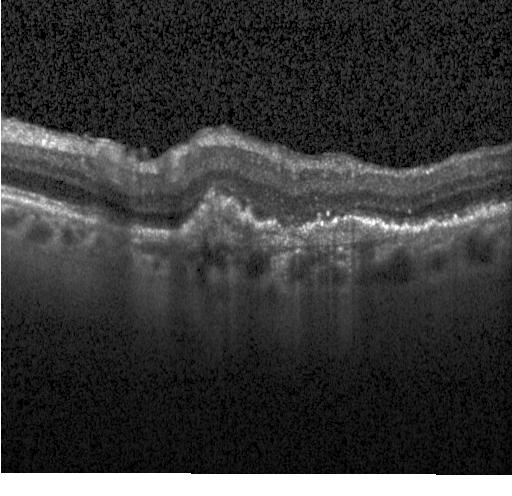
Finding: CNV.